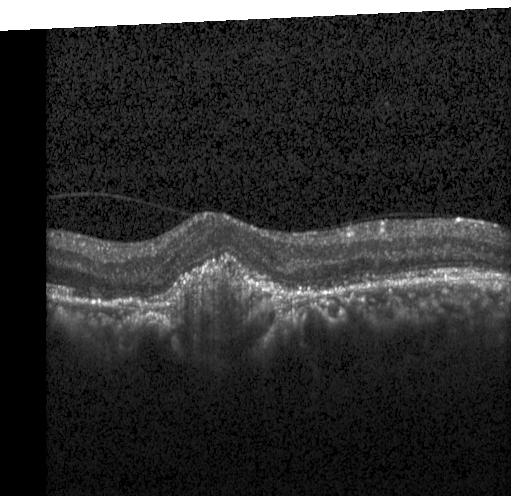 Optical coherence tomography B-scan
Dx: a choroidal neovascular membrane.